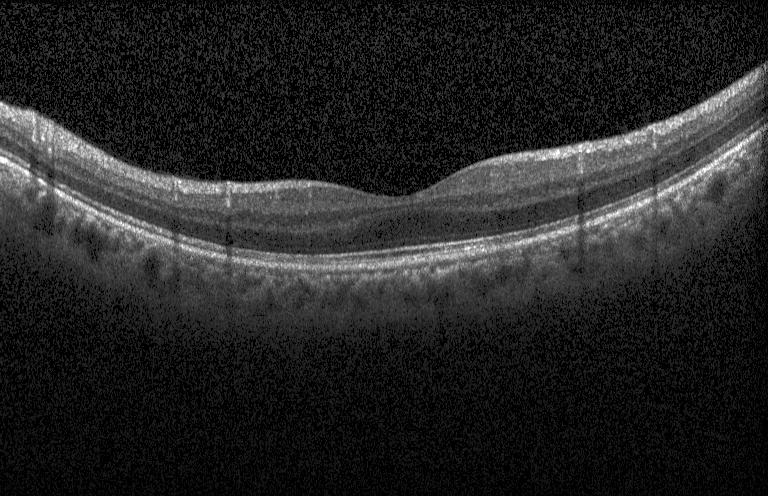

Diagnosis: no evidence of choroidal neovascularization, diabetic macular edema, or drusen.